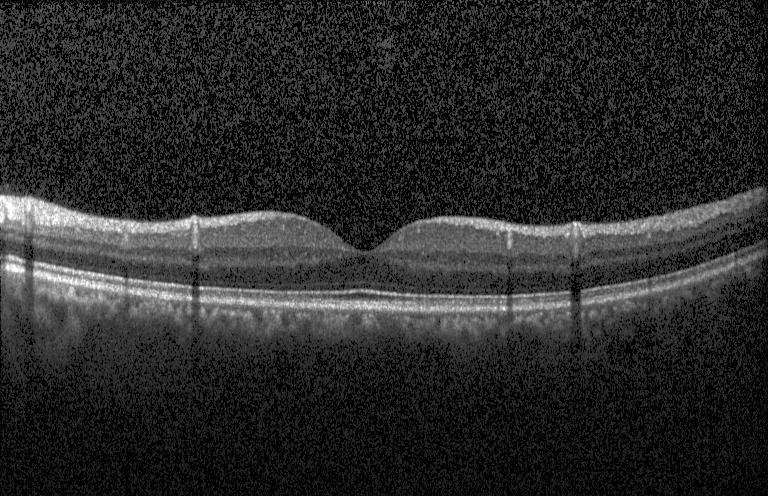

OCT line scan, spectral-domain optical coherence tomography
Dx: no CNV, no DME, and no drusen.